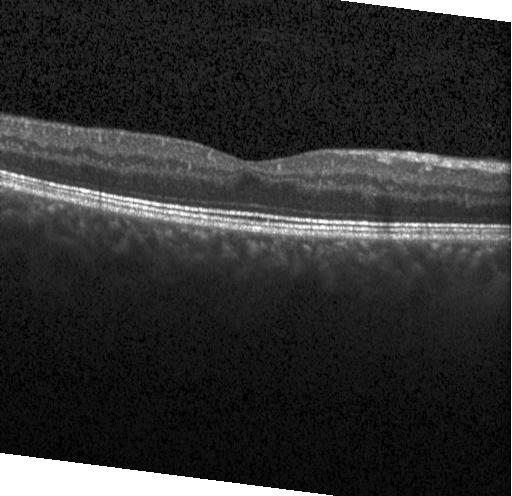 Horizontal scan through the fovea, retinal OCT B-scan. This B-scan demonstrates no CNV, no DME, and no drusen.